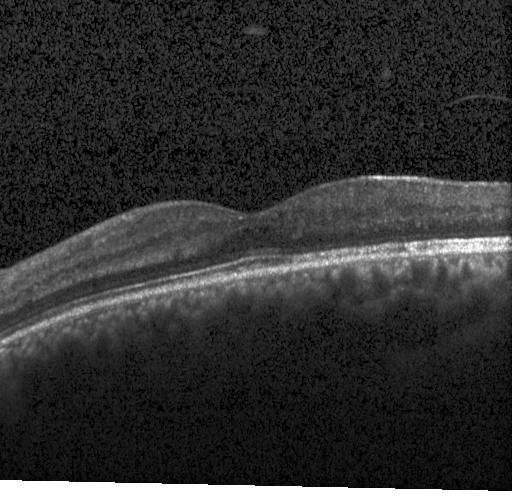 Spectral-domain OCT, optical coherence tomography B-scan, horizontal scan through the fovea, instrument: Heidelberg Spectralis.
Assessment: no choroidal neovascularization, diabetic macular edema, or drusen.